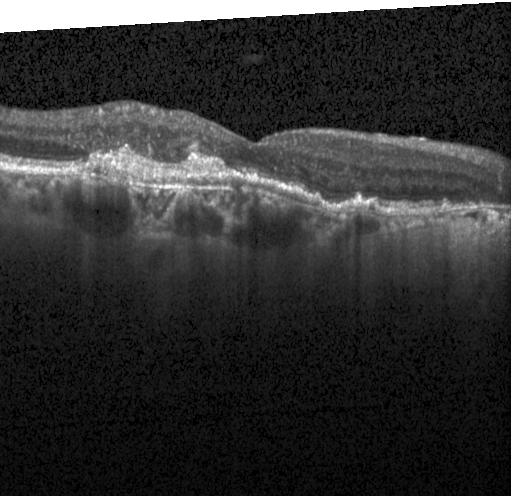
Macular OCT demonstrating choroidal neovascularization.